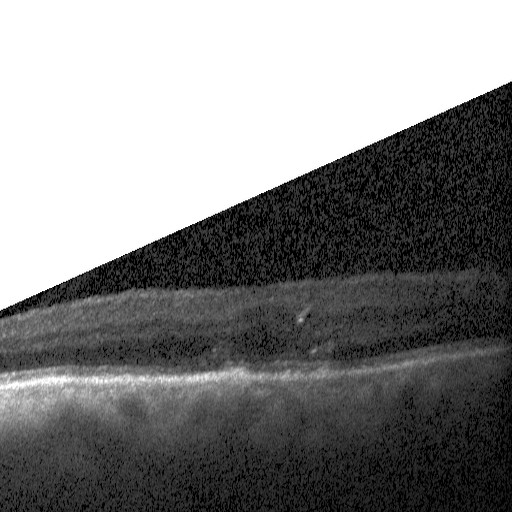

Optical coherence tomography scan, SD-OCT, centered on the fovea
The scan shows diabetic macular edema (DME).